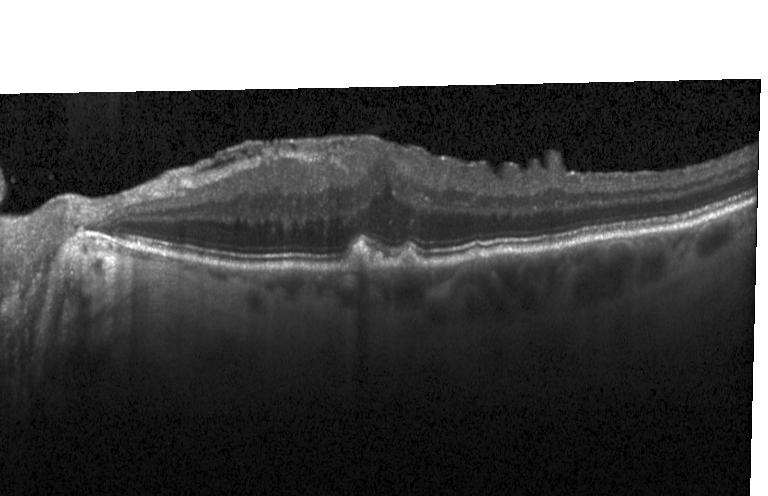
Finding: multiple drusen.